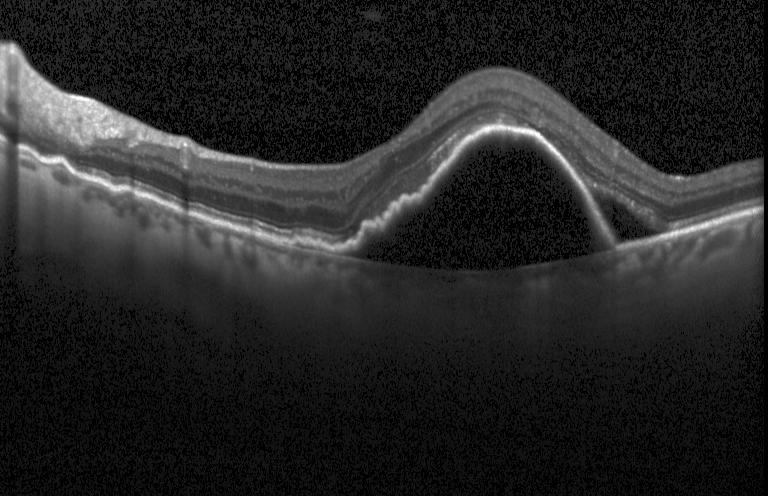

OCT finding: choroidal neovascularization.